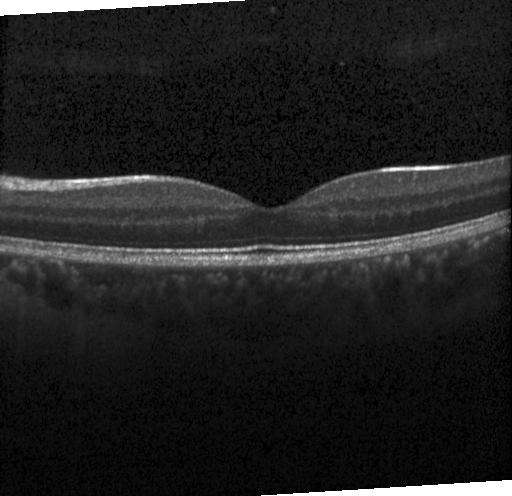

Optical coherence tomography scan, through the macula, spectral-domain OCT, Heidelberg Spectralis OCT system — OCT finding: no CNV, no DME, and no drusen.